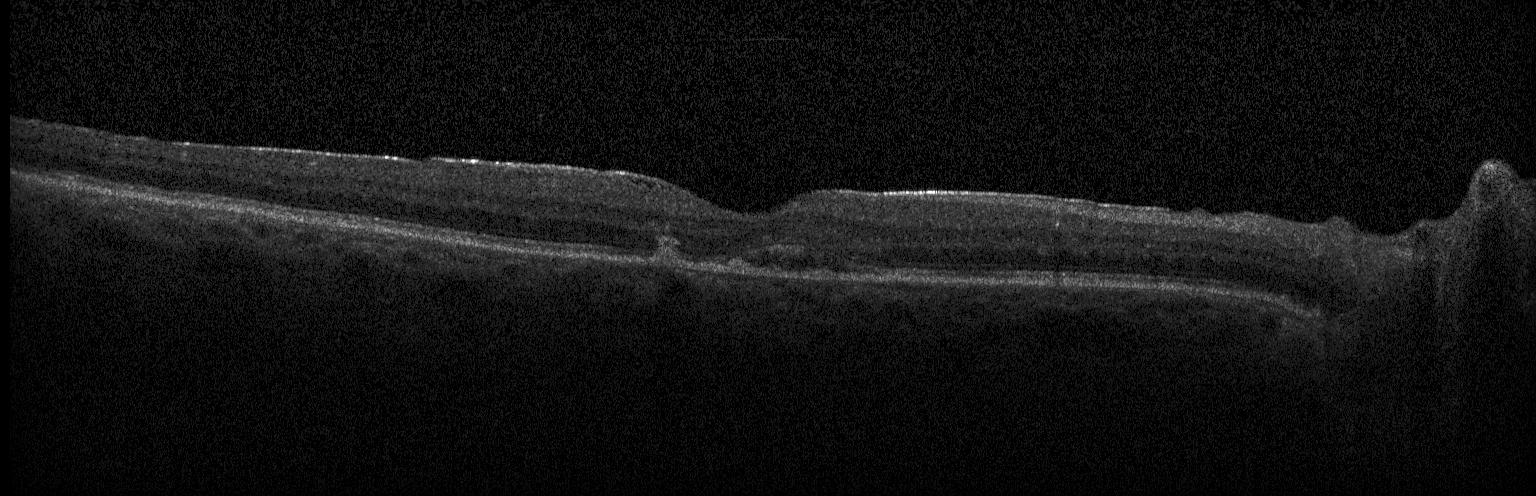

Centered on the fovea. Instrument: Heidelberg Spectralis. Optical coherence tomography scan. Spectral-domain optical coherence tomography.
Finding: choroidal neovascularization.